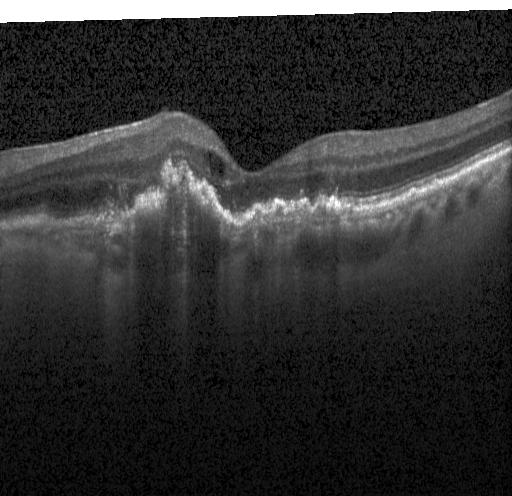
Retinal OCT cross-section.
Diagnosis: a choroidal neovascular membrane.